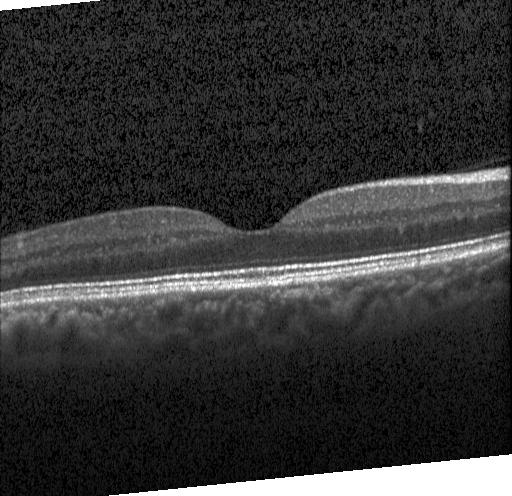
Retinal OCT B-scan; instrument: Heidelberg Spectralis; SD-OCT — Diagnosis: no evidence of choroidal neovascularization, diabetic macular edema, or drusen.